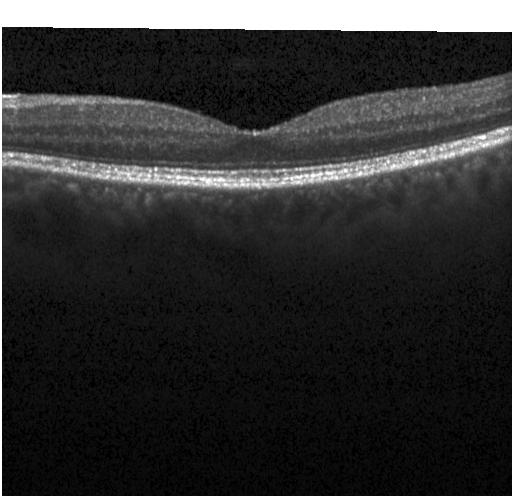
Impression: neither choroidal neovascularization, diabetic macular edema, nor drusen.